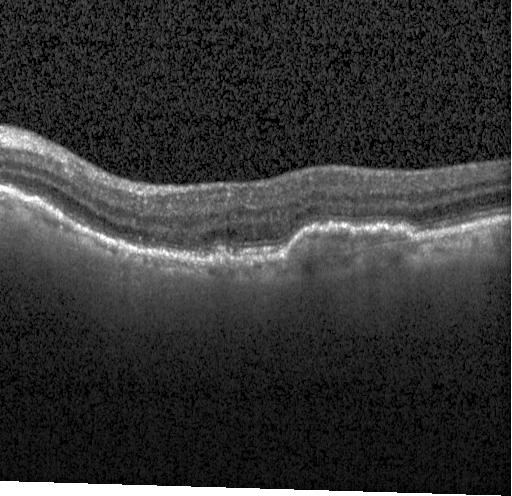
Optical coherence tomography B-scan. Heidelberg Spectralis OCT system. Finding: a choroidal neovascular membrane.